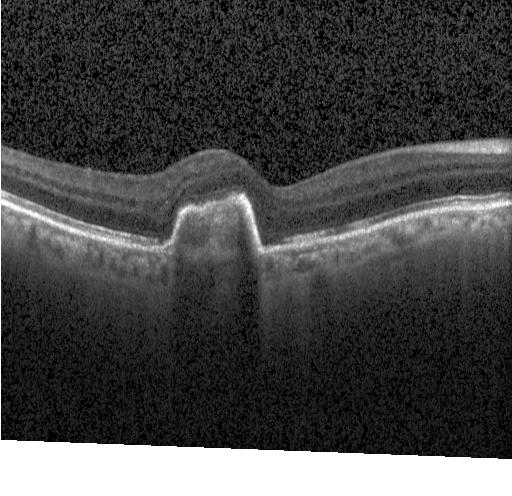
Optical coherence tomography scan, spectral-domain OCT, Heidelberg Spectralis OCT system, macular scan.
This B-scan demonstrates CNV.